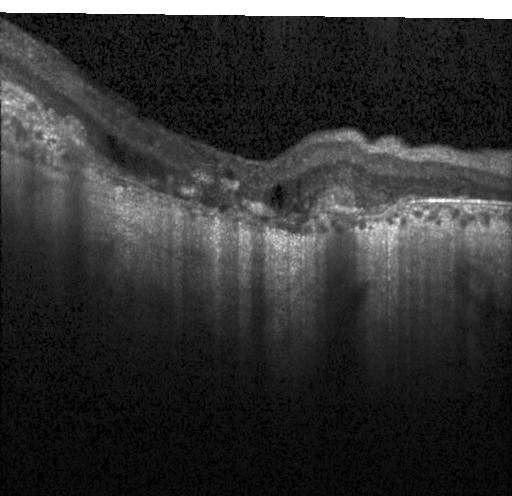 Spectral-domain OCT; macular scan; Heidelberg Spectralis; OCT B-scan.
Finding: a choroidal neovascular membrane.